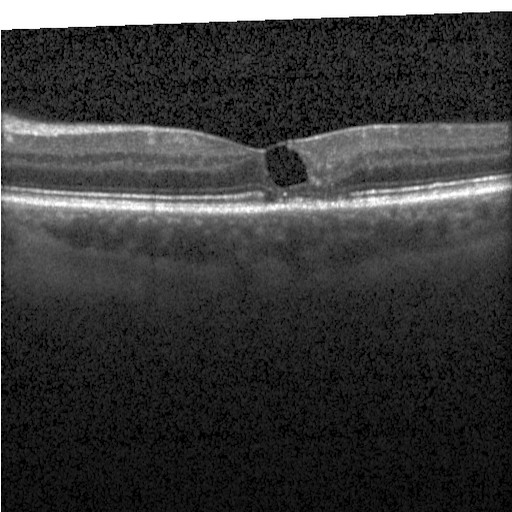 Spectral-domain OCT · acquired on a Heidelberg Spectralis · retinal OCT cross-section · centered on the fovea
The scan shows diabetic macular edema.